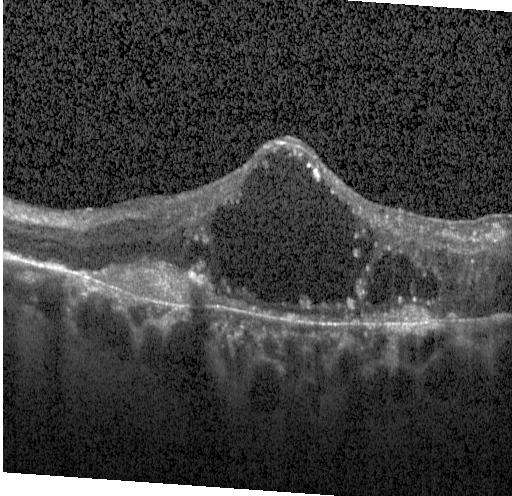 OCT B-scan
A choroidal neovascular membrane.